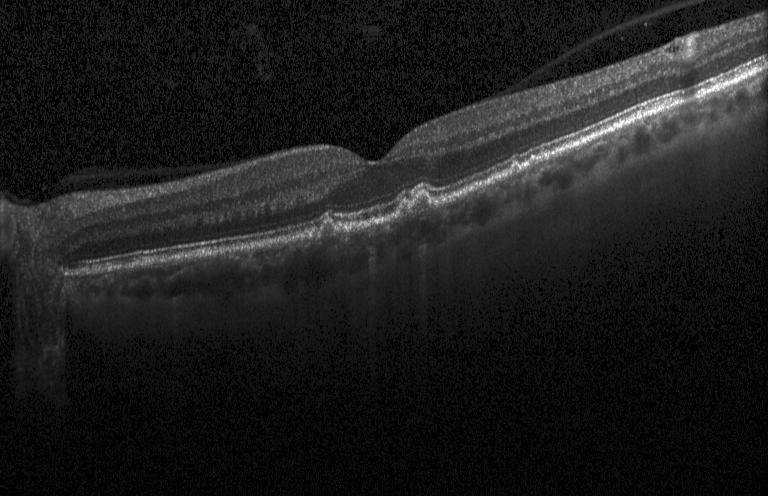

Heidelberg Spectralis; spectral-domain OCT; OCT B-scan; fovea-centered.
Finding: multiple drusen.